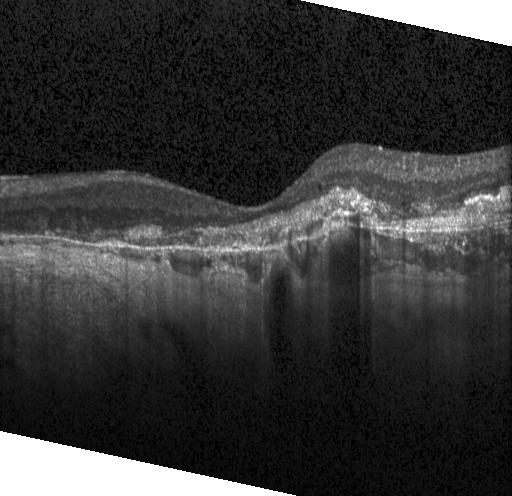

Macular OCT demonstrating choroidal neovascularization.